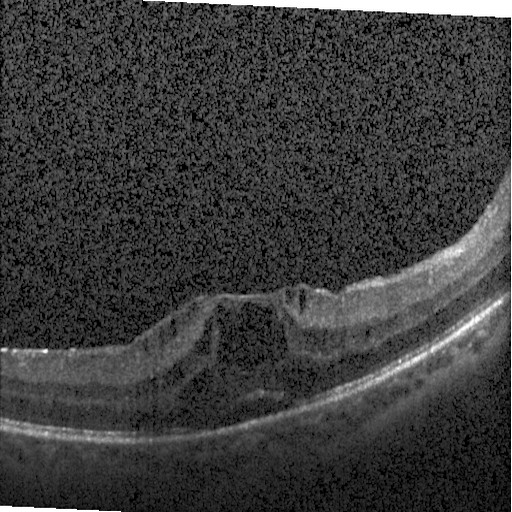
OCT B-scan; acquired on a Heidelberg Spectralis.
Impression: diabetic macular edema.